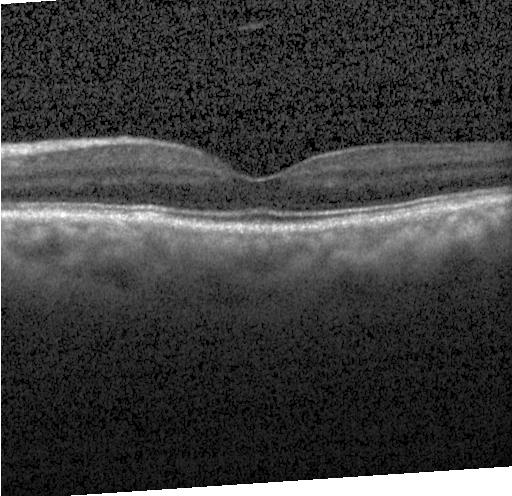
Diagnosis: no choroidal neovascularization, diabetic macular edema, or drusen.